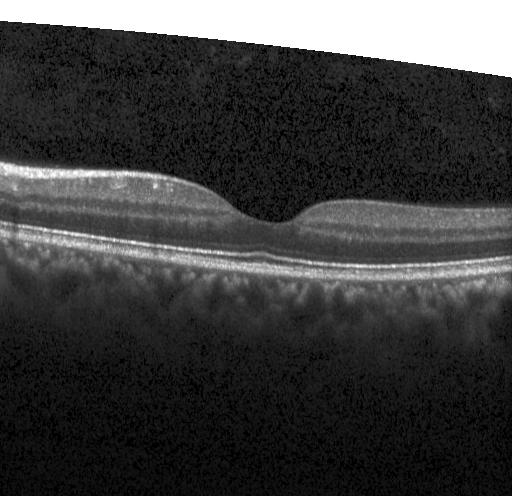 Heidelberg Spectralis · optical coherence tomography scan · through the macula. Impression: no choroidal neovascularization, diabetic macular edema, or drusen.